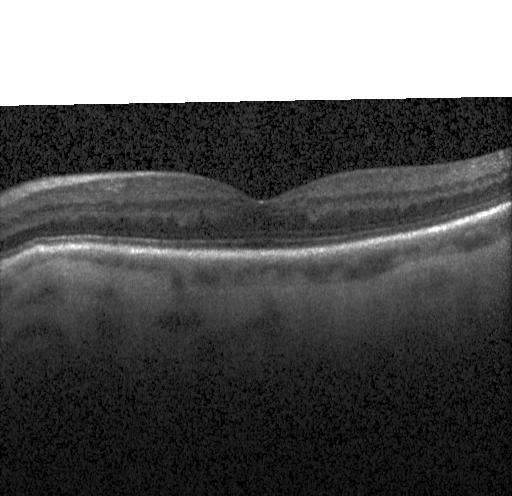 Spectral-domain OCT B-scan: no evidence of choroidal neovascularization, diabetic macular edema, or drusen.